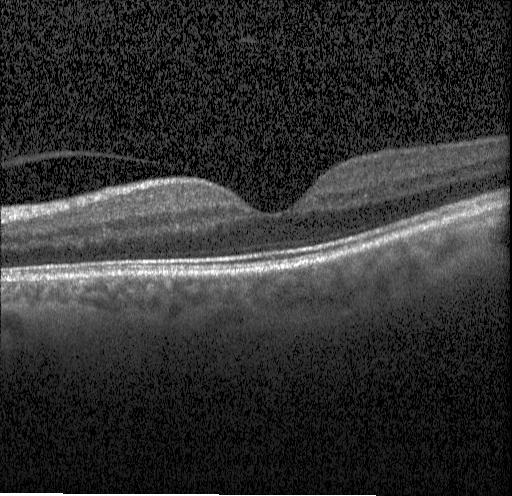

Macular OCT demonstrating no choroidal neovascularization, no diabetic macular edema, and no drusen.